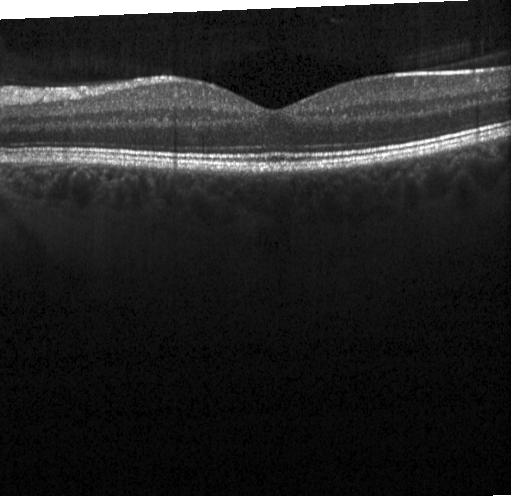
Heidelberg Spectralis OCT system, SD-OCT, optical coherence tomography scan, fovea-centered.
Assessment: no evidence of choroidal neovascularization, diabetic macular edema, or drusen.